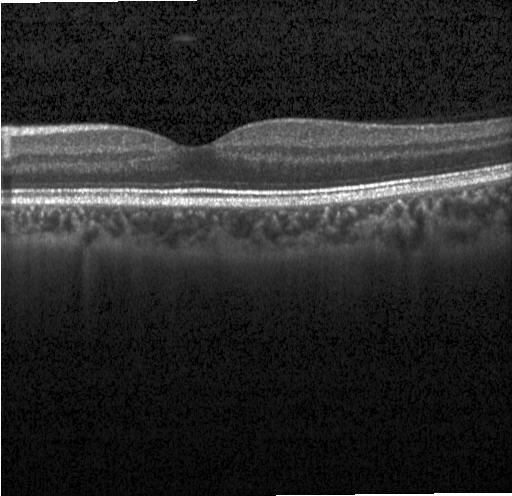 Macular OCT demonstrating no choroidal neovascularization, diabetic macular edema, or drusen.